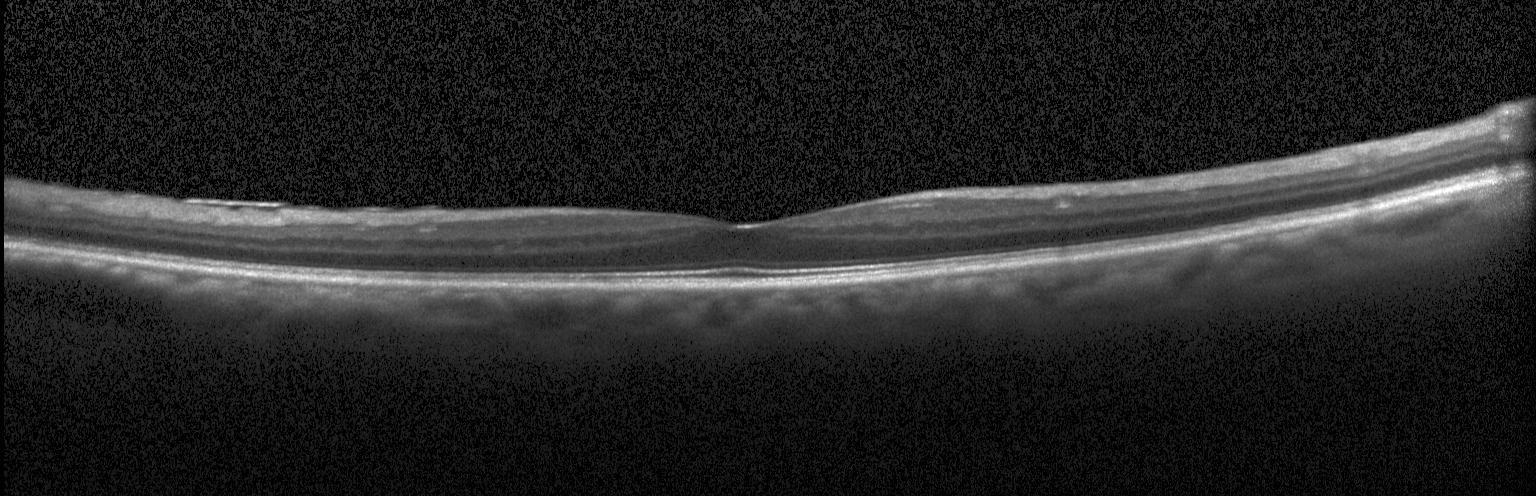

Spectral-domain OCT B-scan: no choroidal neovascularization, no diabetic macular edema, and no drusen.